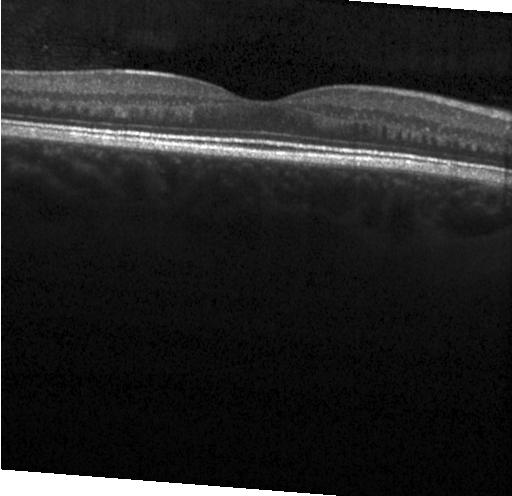

Optical coherence tomography scan. Finding: no choroidal neovascularization, no diabetic macular edema, and no drusen.